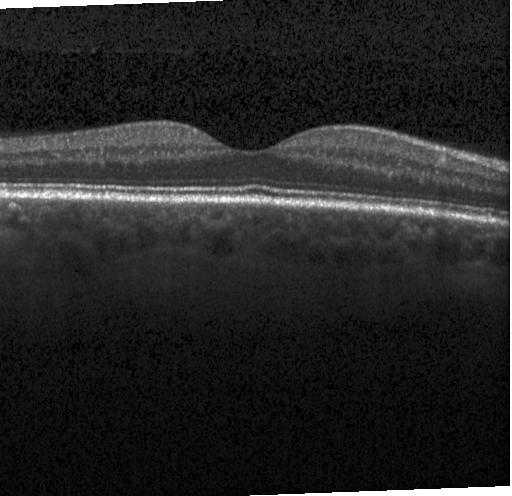
Finding: no choroidal neovascularization, no diabetic macular edema, and no drusen.